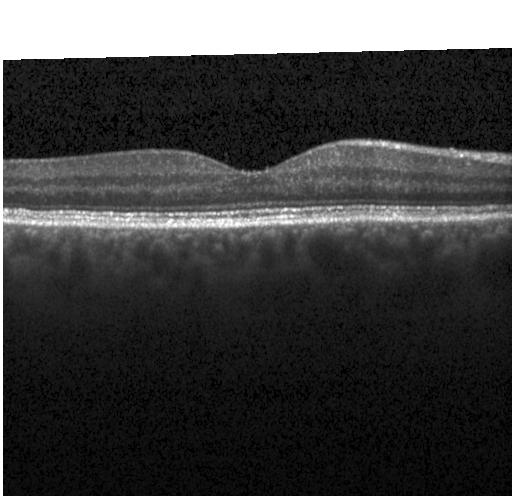 Macular OCT demonstrating neither choroidal neovascularization, diabetic macular edema, nor drusen.